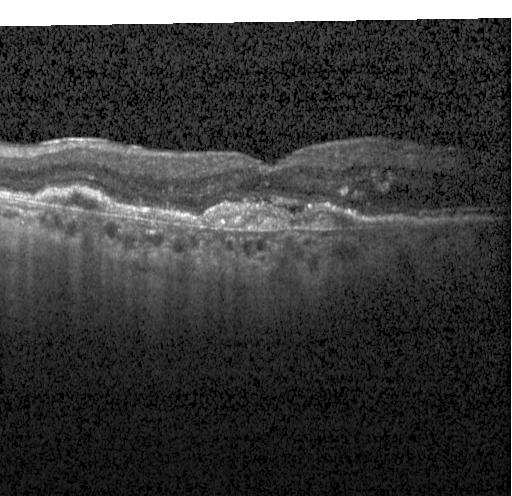
Heidelberg Spectralis OCT system, retinal OCT B-scan
Diagnosis: choroidal neovascularization.